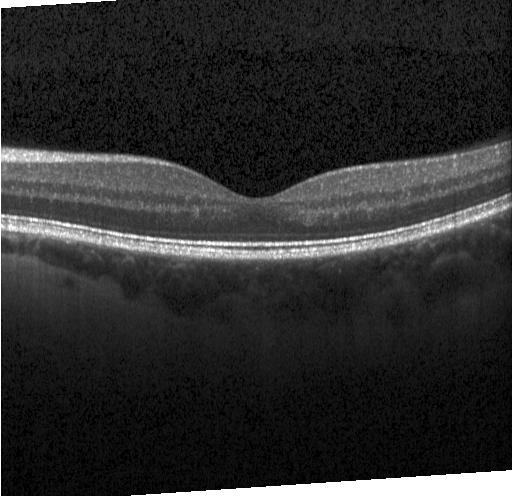
OCT finding: no evidence of CNV, DME, or drusen.